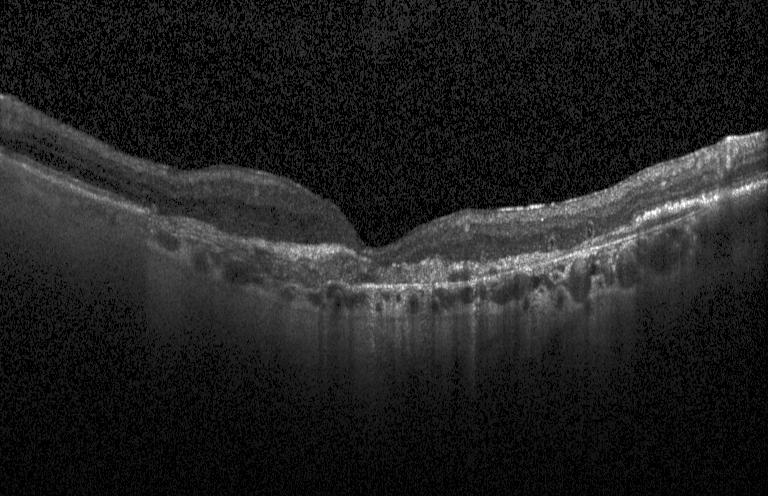 OCT B-scan showing choroidal neovascularization.